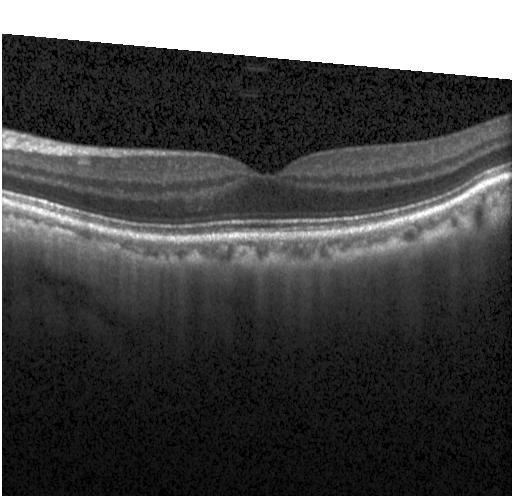

Neither choroidal neovascularization, diabetic macular edema, nor drusen.